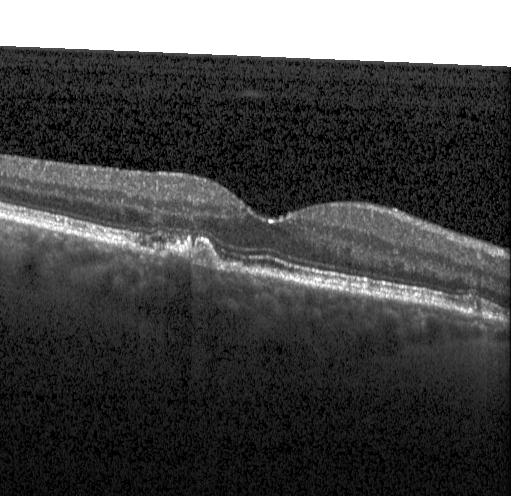
Diagnosis: choroidal neovascularization.